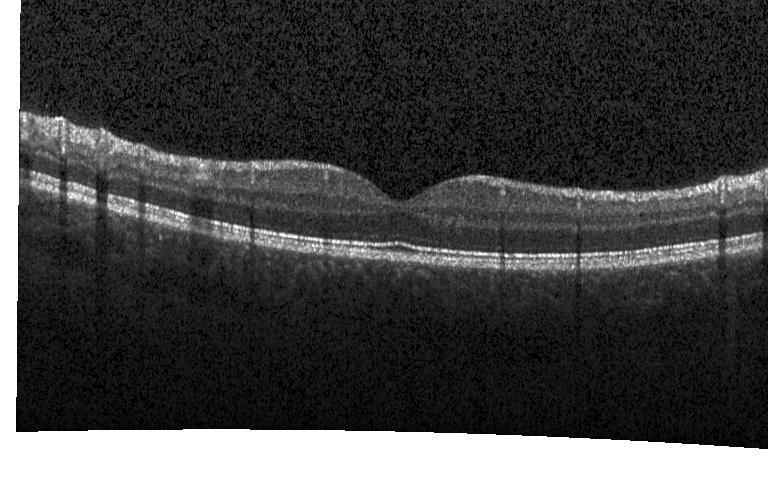
Retinal OCT cross-section
No choroidal neovascularization, diabetic macular edema, or drusen.